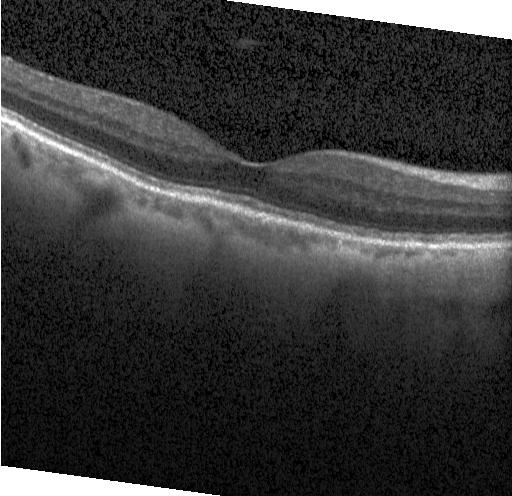 Retinal OCT cross-section — Impression: neither choroidal neovascularization, diabetic macular edema, nor drusen.